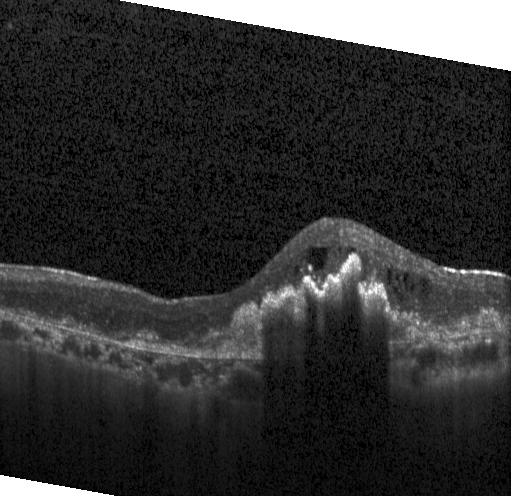 Macular OCT demonstrating a choroidal neovascular membrane.